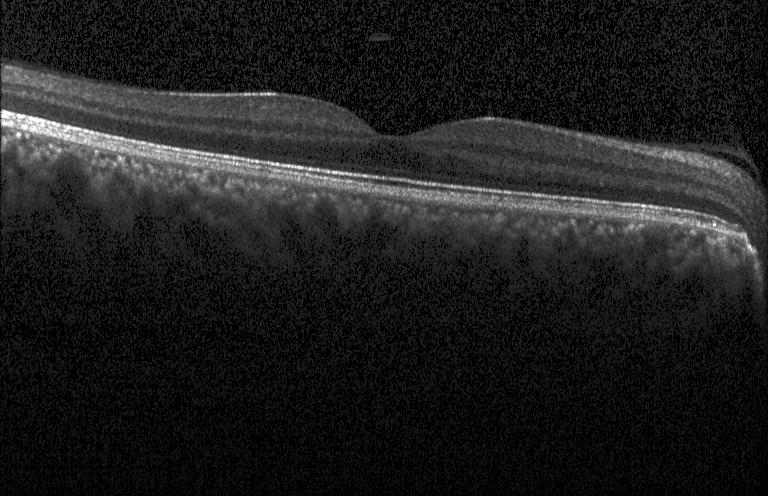

Retinal OCT B-scan, acquired on a Heidelberg Spectralis. Dx: no choroidal neovascularization, diabetic macular edema, or drusen.